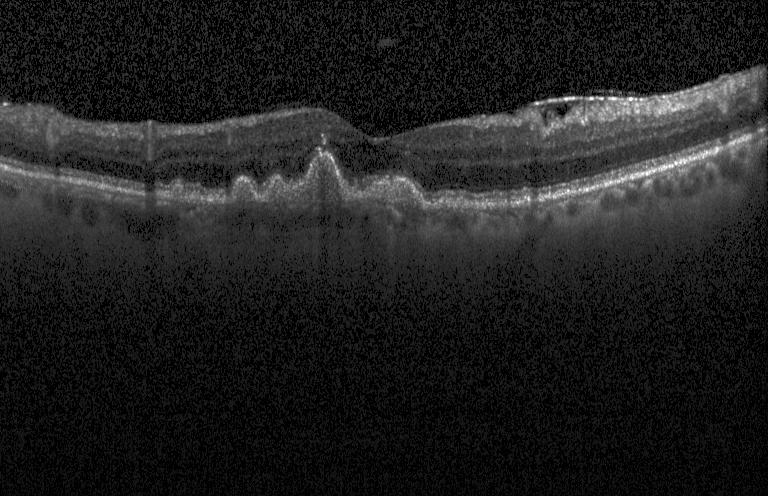
OCT scan showing a choroidal neovascular membrane.